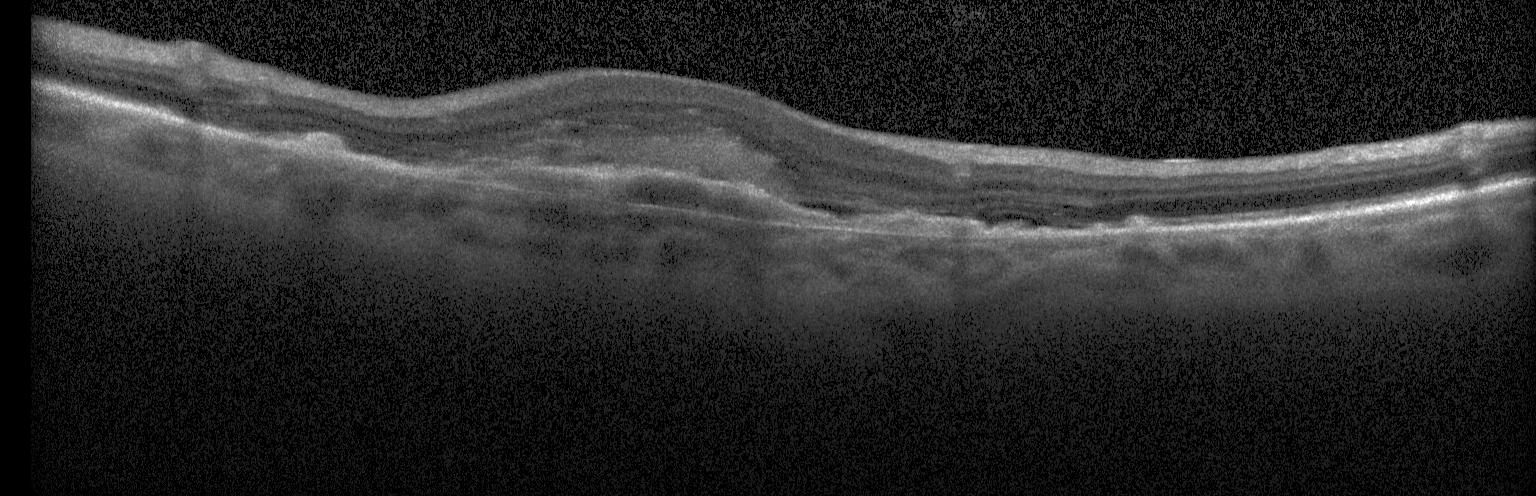
Finding: choroidal neovascularization.